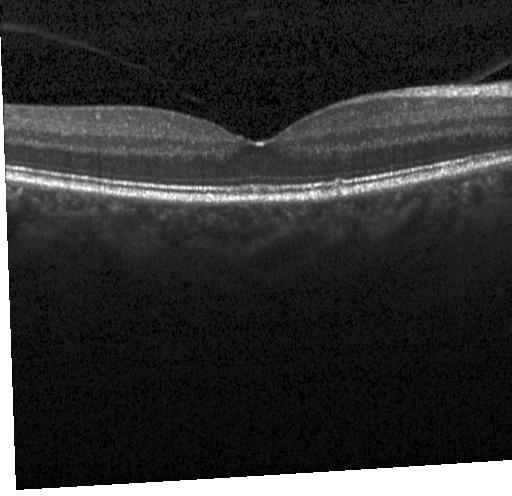

Spectral-domain optical coherence tomography. Optical coherence tomography B-scan. Heidelberg Spectralis
Diagnosis: sub-RPE drusenoid deposits.